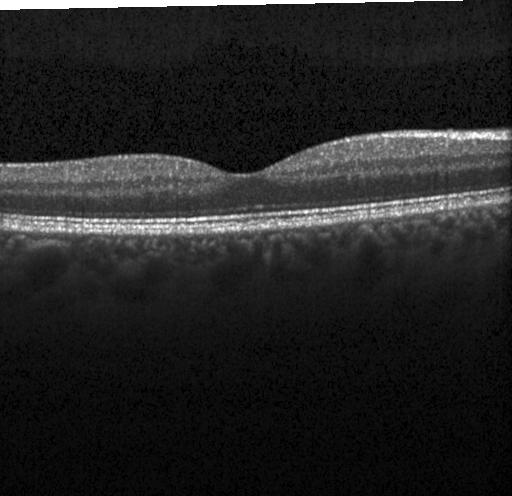
Optical coherence tomography scan; spectral-domain optical coherence tomography; fovea-centered — No choroidal neovascularization, diabetic macular edema, or drusen.